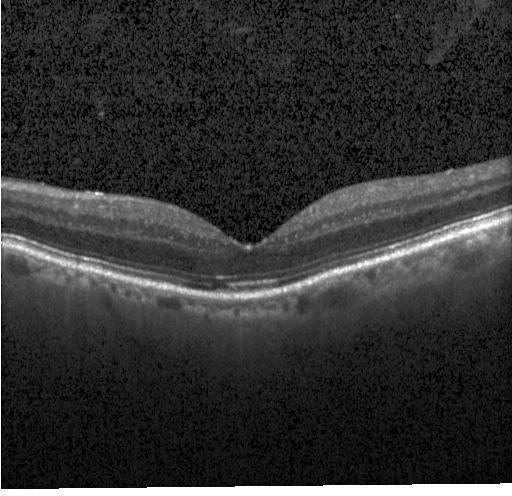 The scan shows neither CNV, DME, nor drusen.